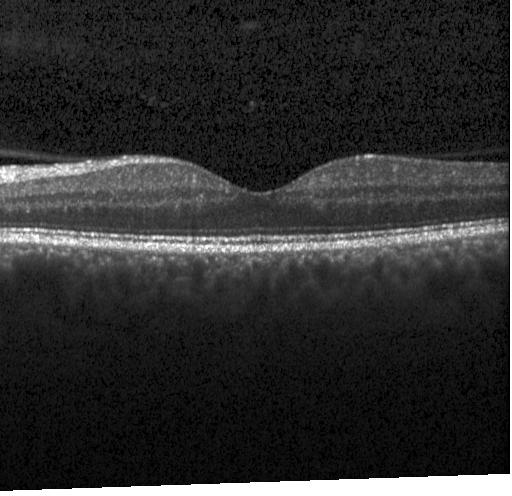
Diagnosis: neither choroidal neovascularization, diabetic macular edema, nor drusen.